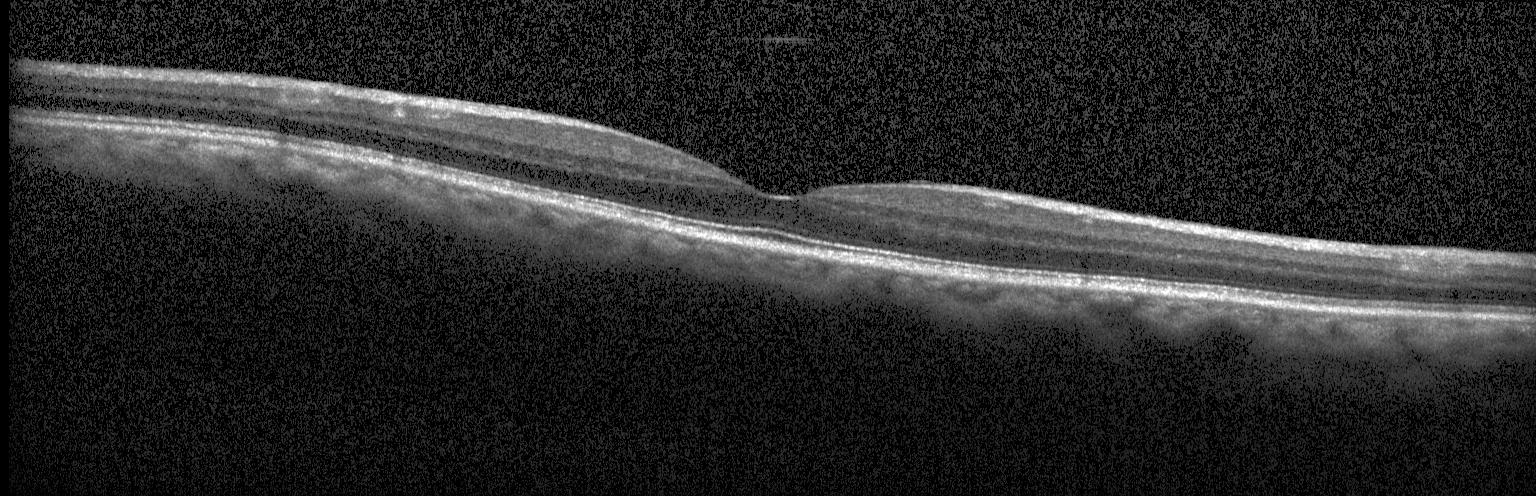
Macular OCT: no choroidal neovascularization, no diabetic macular edema, and no drusen.